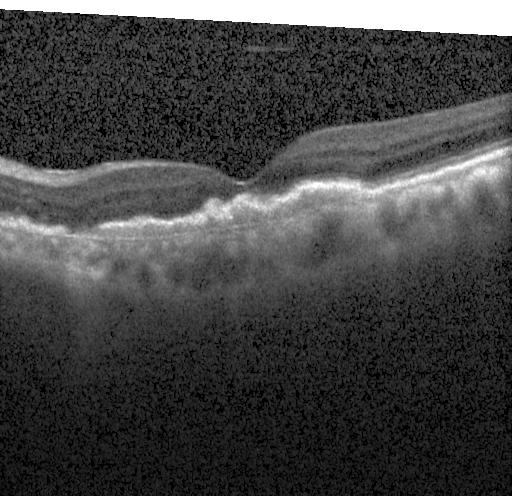 Retinal OCT cross-section; spectral-domain OCT; centered on the fovea; acquired on a Heidelberg Spectralis
Dx: a choroidal neovascular membrane.